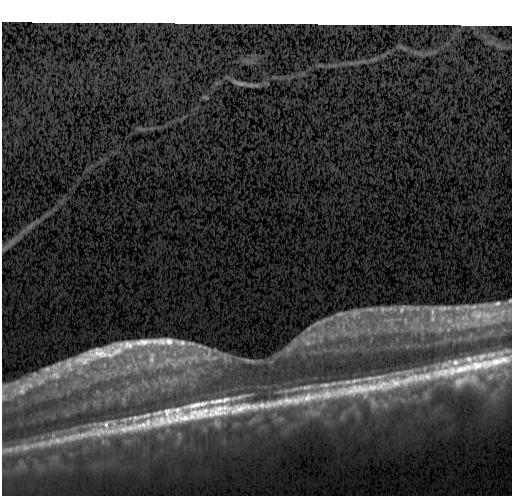
This B-scan demonstrates neither choroidal neovascularization, diabetic macular edema, nor drusen.